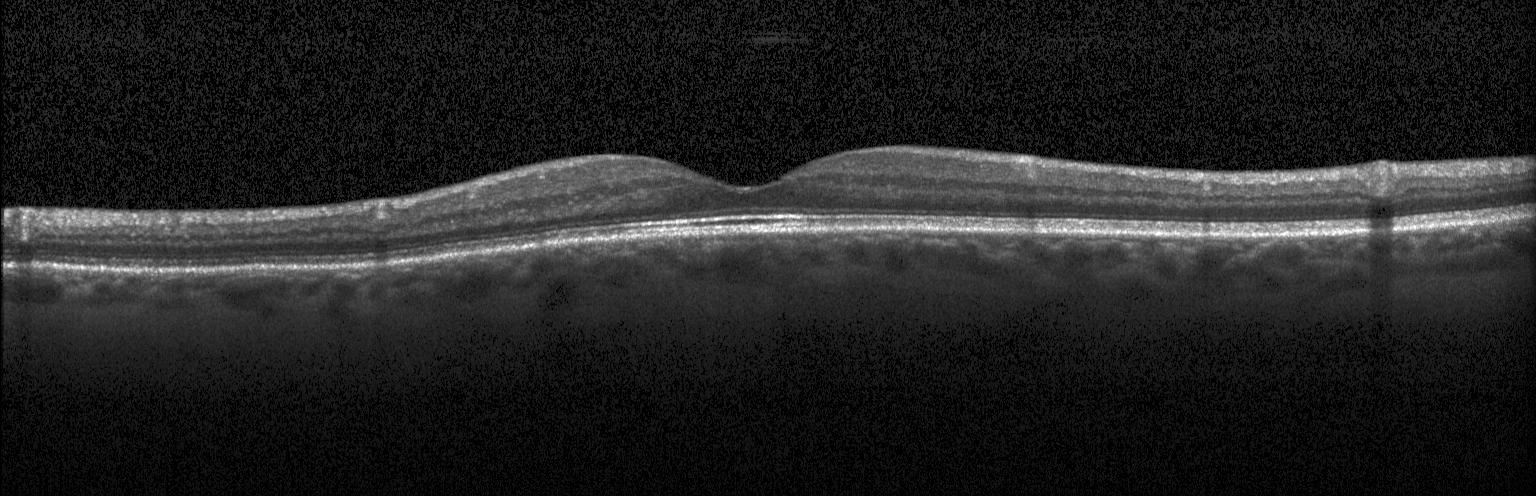 Acquired on a Heidelberg Spectralis. Spectral-domain optical coherence tomography. OCT line scan. Diagnosis: no CNV, DME, or drusen.